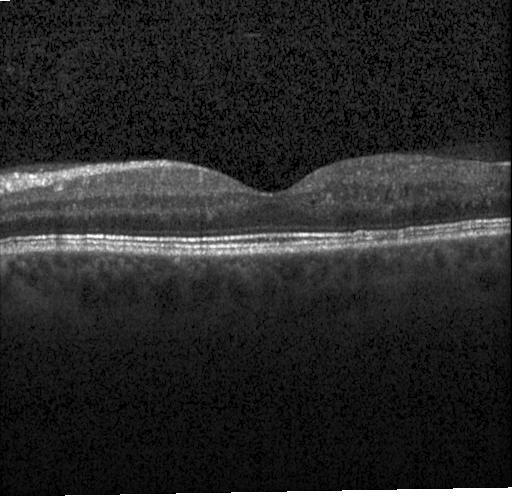

Retinal OCT cross-section showing neither choroidal neovascularization, diabetic macular edema, nor drusen.